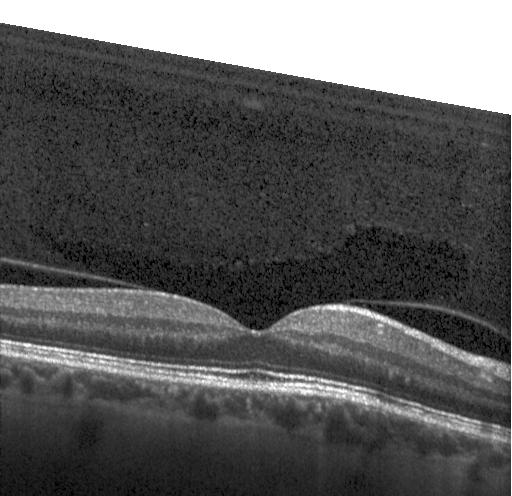 Centered on the fovea · spectral-domain OCT · optical coherence tomography B-scan
Finding: no choroidal neovascularization, diabetic macular edema, or drusen.